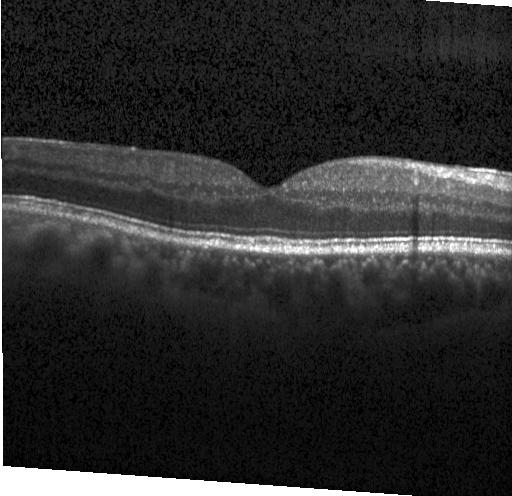
Spectral-domain OCT B-scan: no choroidal neovascularization, no diabetic macular edema, and no drusen.